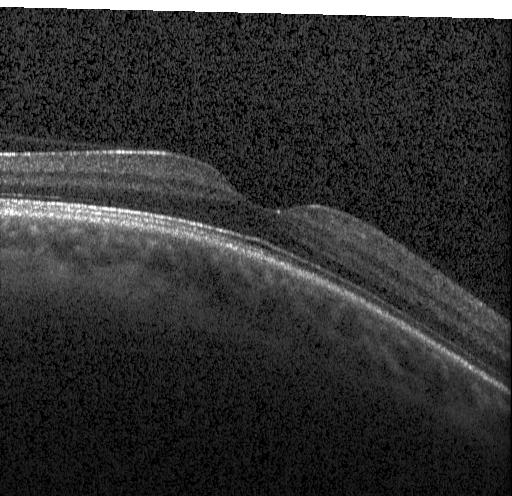

Retinal OCT cross-section — Macular OCT: neither choroidal neovascularization, diabetic macular edema, nor drusen.